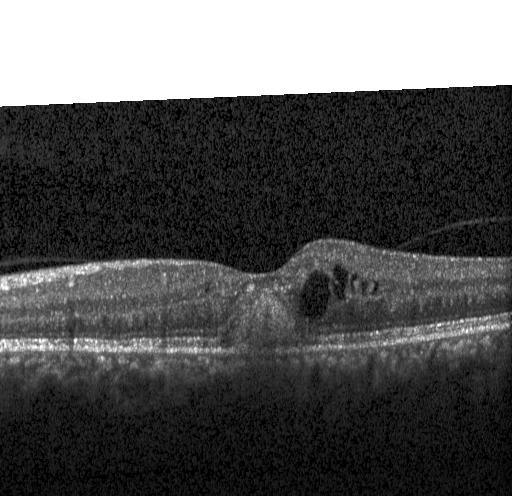

Heidelberg Spectralis · OCT line scan · fovea-centered
Impression: CNV.